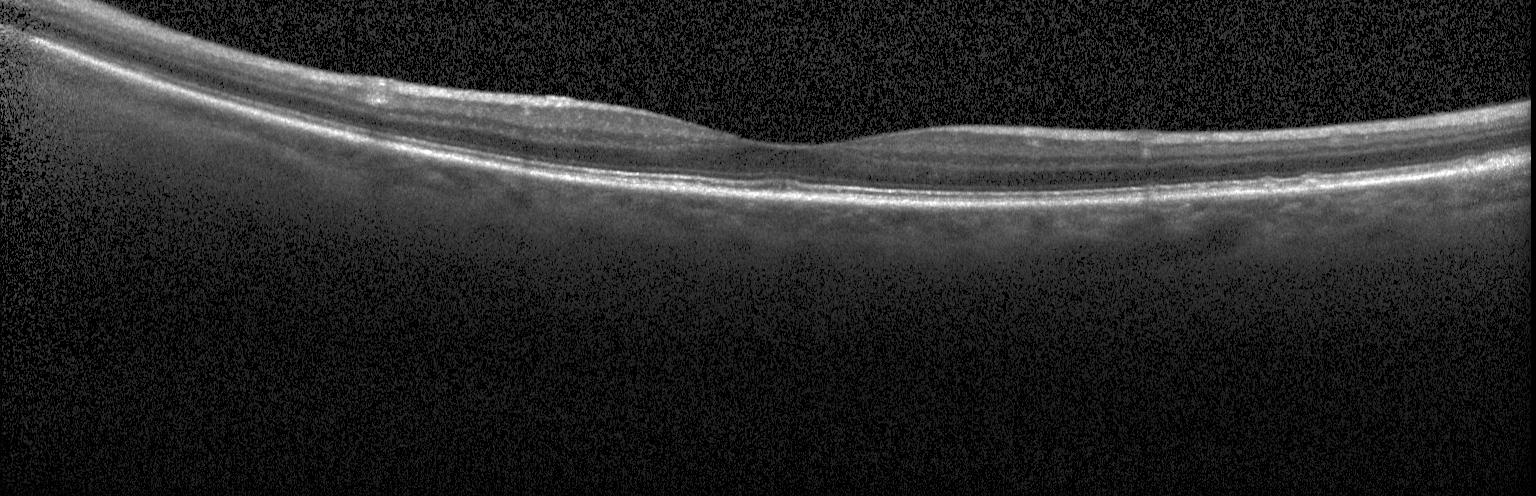
Heidelberg Spectralis OCT system. Horizontal scan through the fovea. Retinal OCT B-scan
Assessment: neither choroidal neovascularization, diabetic macular edema, nor drusen.